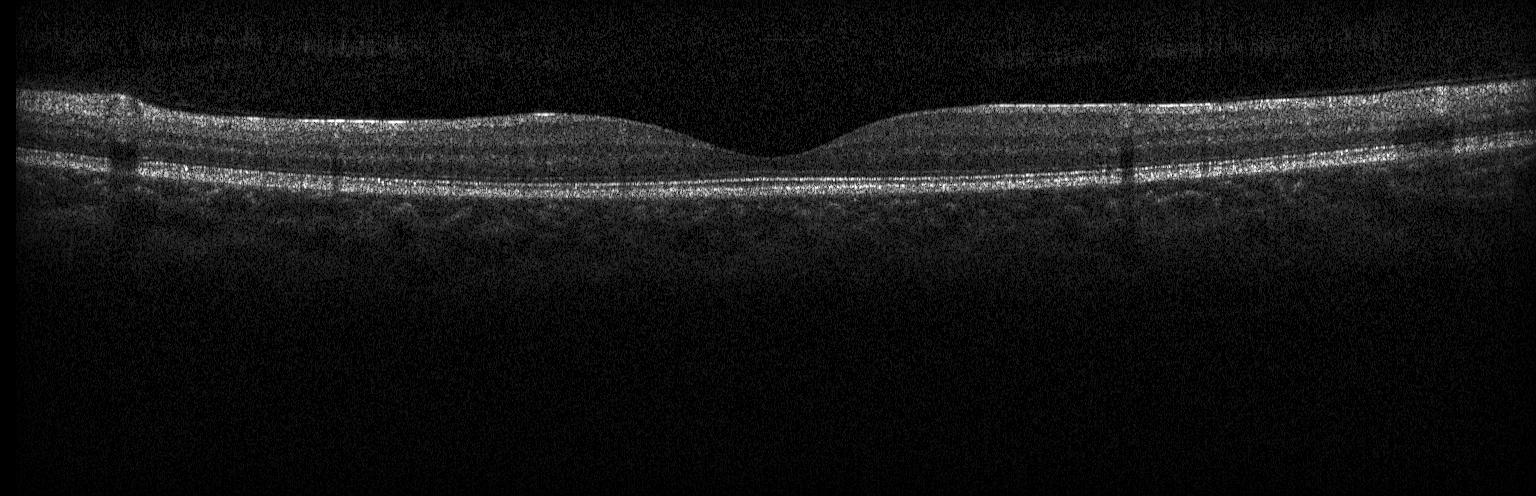 Assessment: no choroidal neovascularization, diabetic macular edema, or drusen.